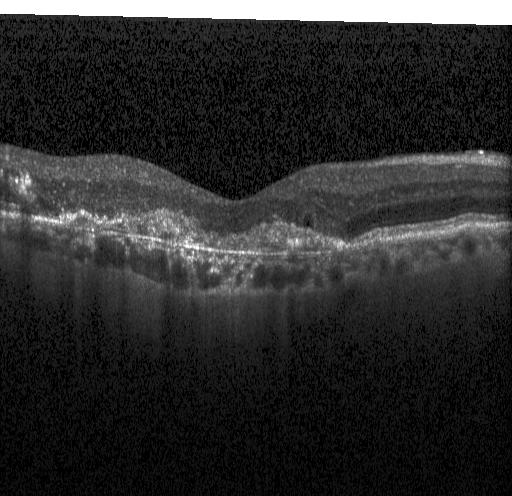
OCT B-scan. Heidelberg Spectralis. Diagnosis: CNV.